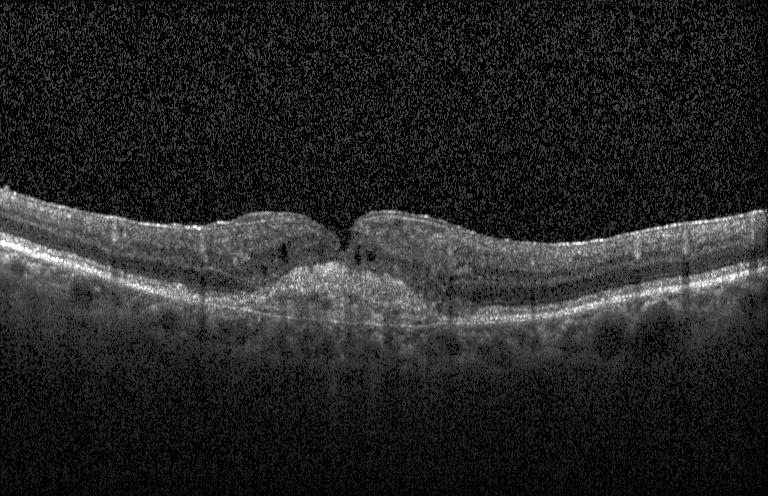 OCT B-scan showing choroidal neovascularization (CNV).